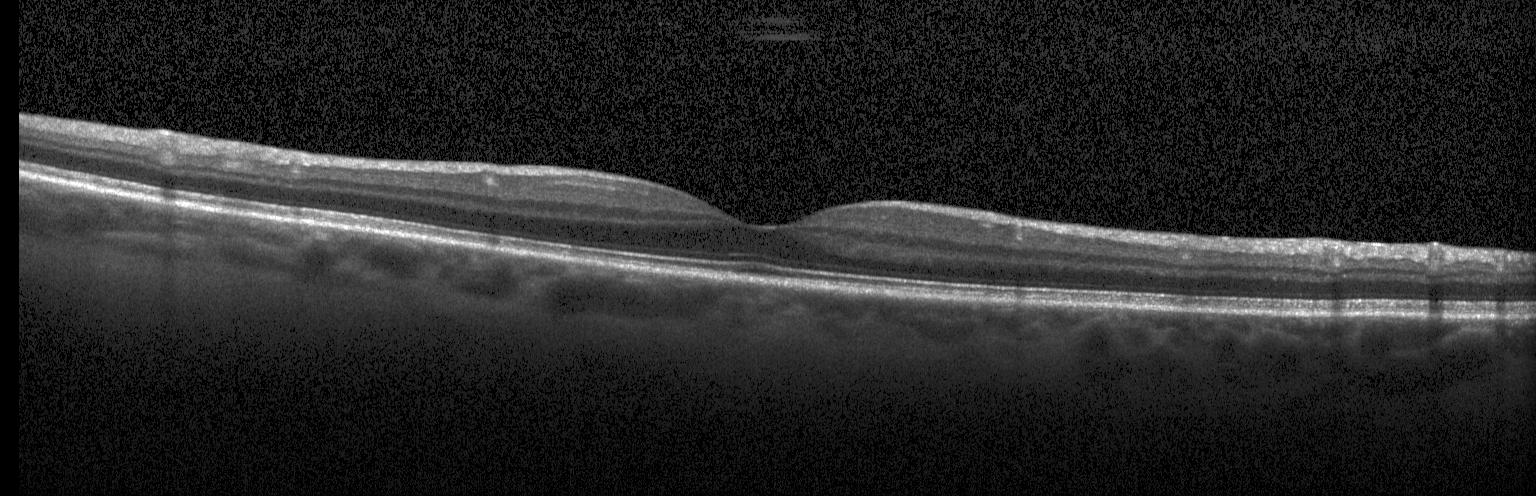
SD-OCT, Heidelberg Spectralis, optical coherence tomography scan, through the macula.
Impression: no evidence of choroidal neovascularization, diabetic macular edema, or drusen.